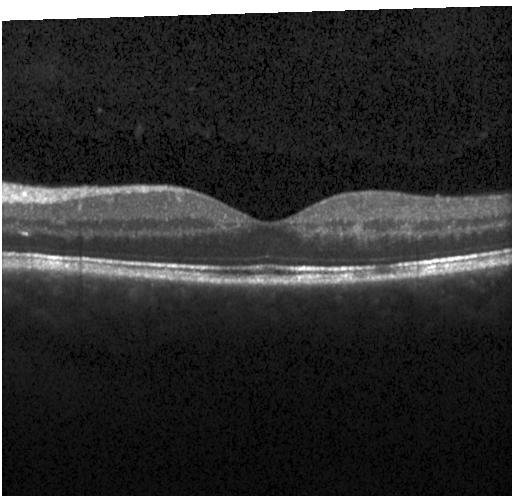 Optical coherence tomography B-scan · macular scan · instrument: Heidelberg Spectralis · spectral-domain OCT.
Impression: neither CNV, DME, nor drusen.